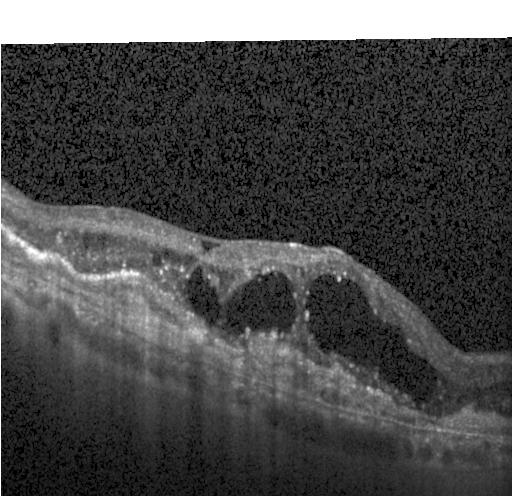 Spectral-domain optical coherence tomography. Instrument: Heidelberg Spectralis. Optical coherence tomography B-scan.
A choroidal neovascular membrane.